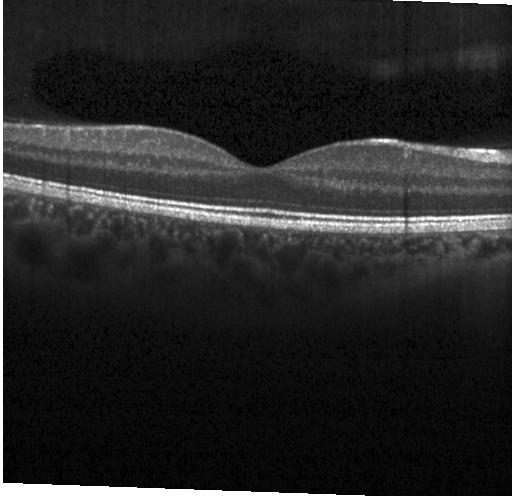

Diagnosis: no evidence of choroidal neovascularization, diabetic macular edema, or drusen.